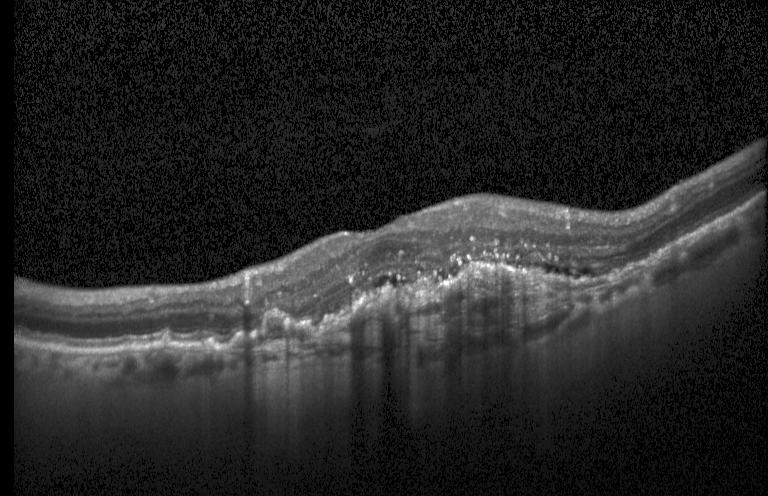 Heidelberg Spectralis OCT system, SD-OCT, retinal OCT B-scan, horizontal scan through the fovea. Impression: choroidal neovascularization (CNV).